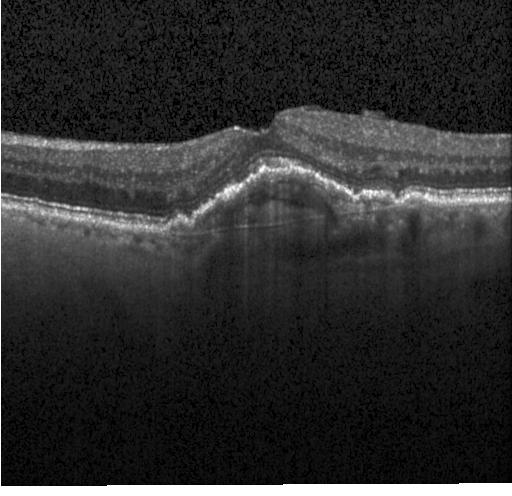

Through the macula. Retinal OCT B-scan. Instrument: Heidelberg Spectralis. OCT finding: a choroidal neovascular membrane.